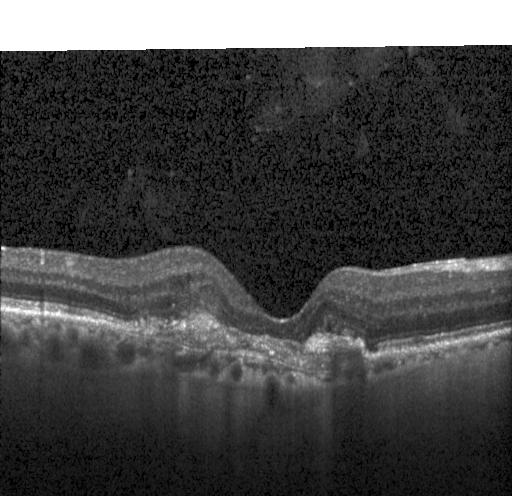 Dx: choroidal neovascularization.